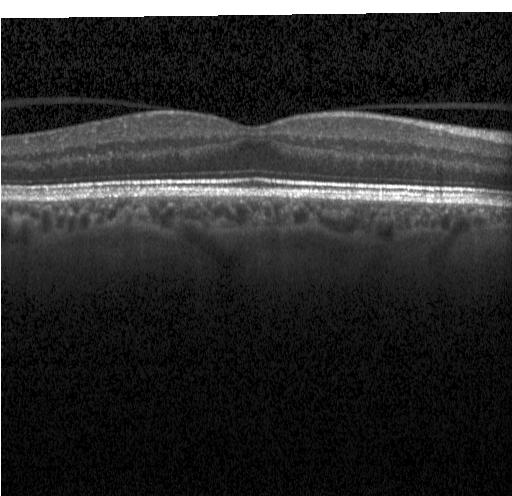

Spectral-domain OCT · fovea-centered · OCT line scan — Finding: no CNV, DME, or drusen.